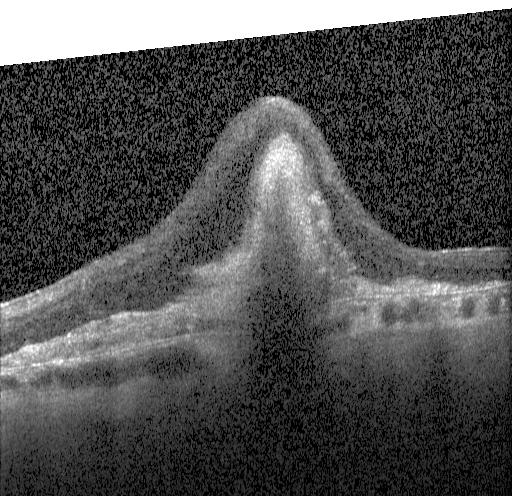
Optical coherence tomography B-scan — Finding: a choroidal neovascular membrane.